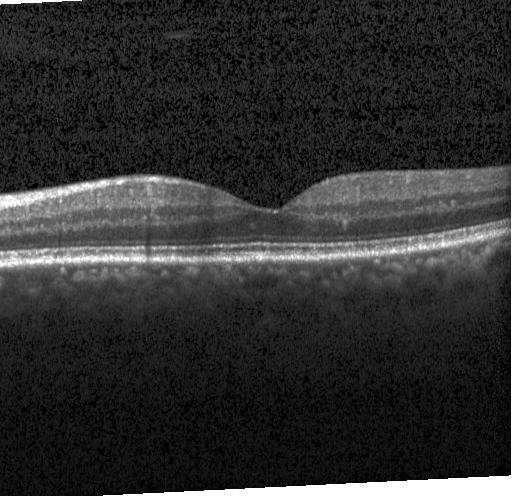

Diagnosis: no evidence of choroidal neovascularization, diabetic macular edema, or drusen.